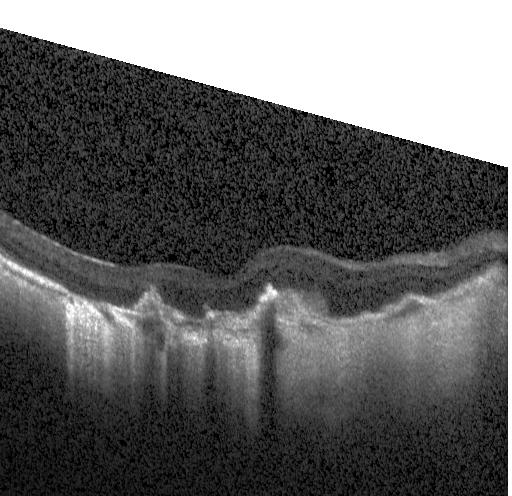
Centered on the fovea; Heidelberg Spectralis; spectral-domain optical coherence tomography; OCT B-scan — The scan shows choroidal neovascularization (CNV).